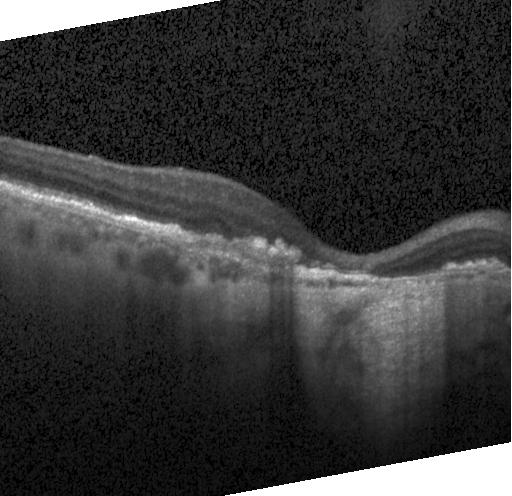

OCT line scan. OCT finding: choroidal neovascularization (CNV).